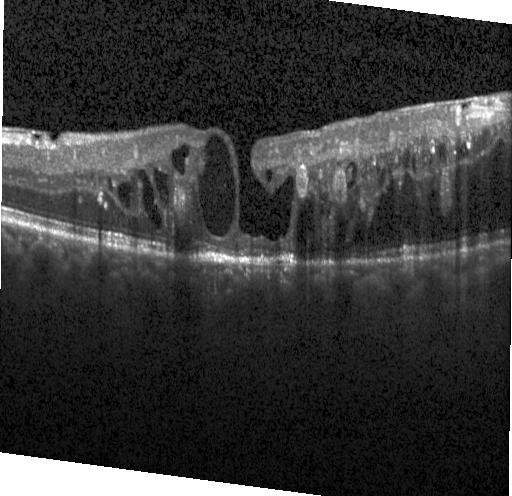

Heidelberg Spectralis OCT system. Optical coherence tomography scan. Macular scan. SD-OCT — The scan shows diabetic macular edema (DME).